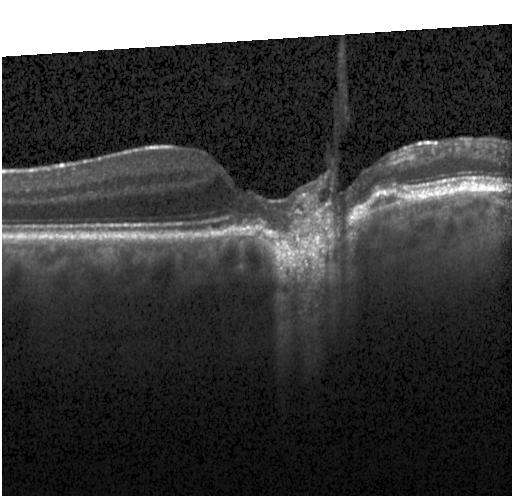

OCT B-scan — Impression: a choroidal neovascular membrane.